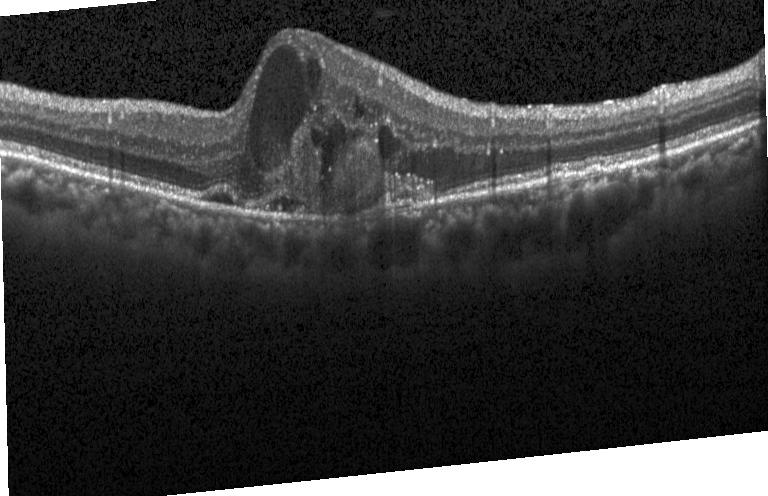 Finding: choroidal neovascularization (CNV).